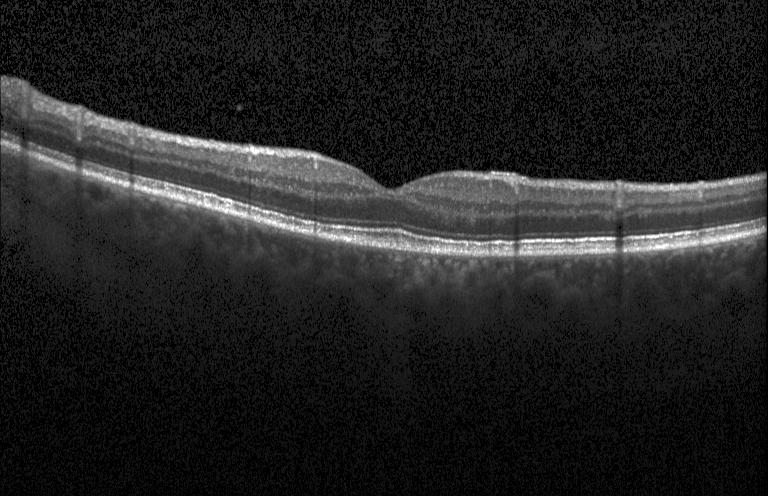 Diagnosis: neither choroidal neovascularization, diabetic macular edema, nor drusen.